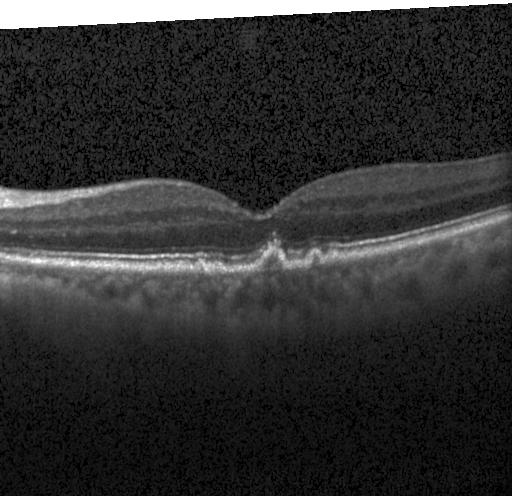
OCT B-scan.
This B-scan demonstrates sub-RPE drusenoid deposits.